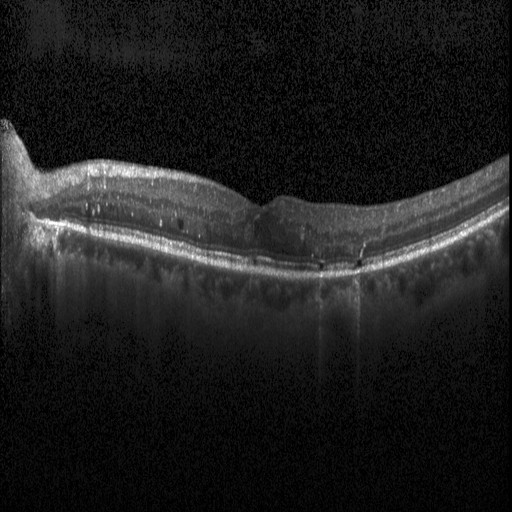 This B-scan demonstrates diabetic macular edema (DME).